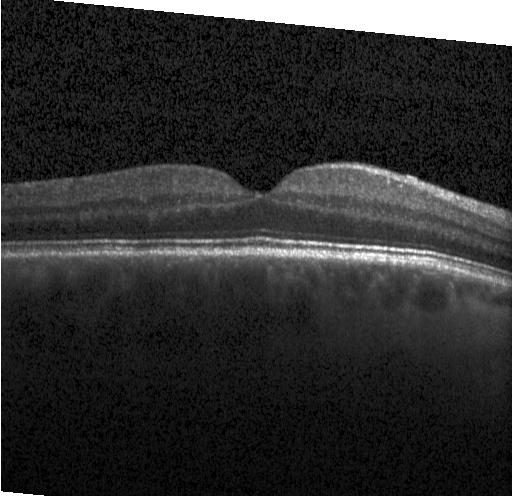 Impression: no evidence of choroidal neovascularization, diabetic macular edema, or drusen.